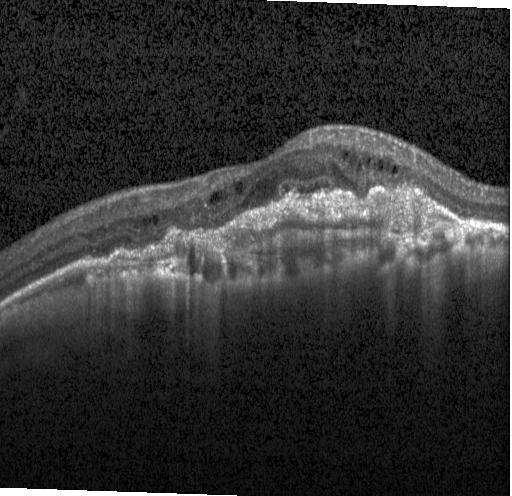
OCT B-scan. Diagnosis: choroidal neovascularization.